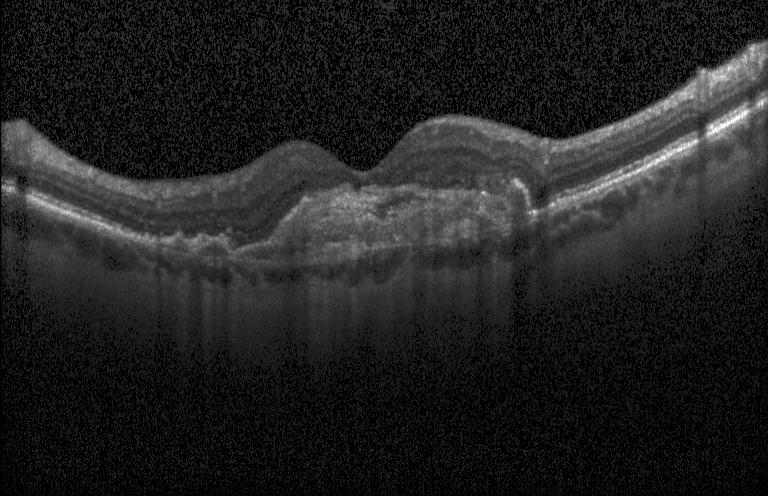
This B-scan demonstrates a choroidal neovascular membrane.